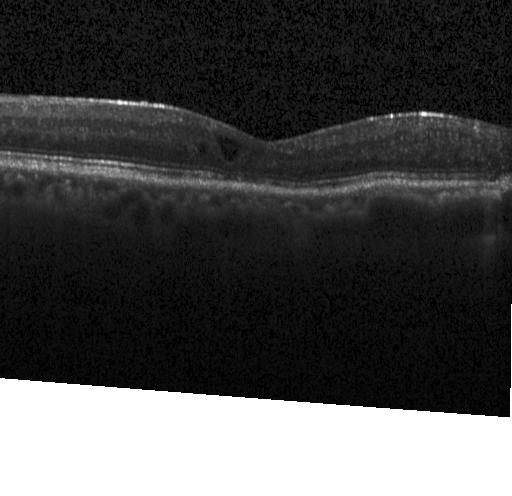
Diabetic macular edema.